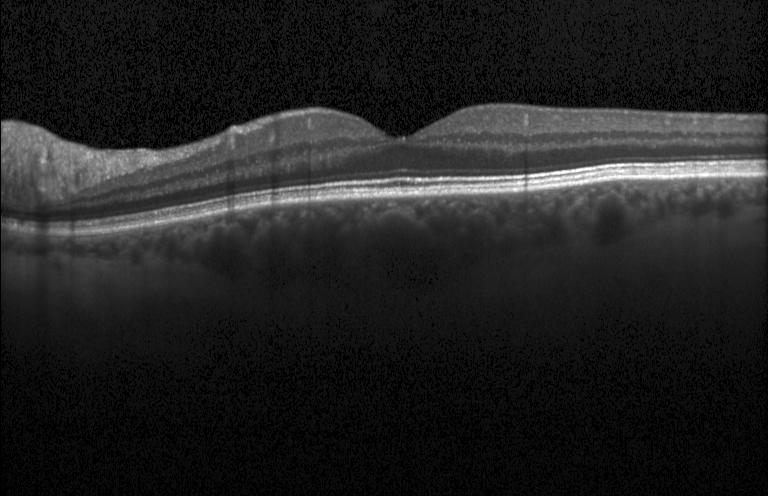

Through the macula; OCT B-scan; Heidelberg Spectralis OCT system
This B-scan demonstrates no choroidal neovascularization, diabetic macular edema, or drusen.